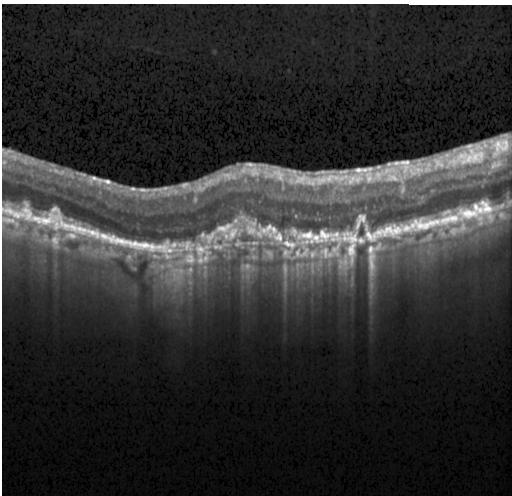
Macular scan, optical coherence tomography B-scan
The scan shows CNV.